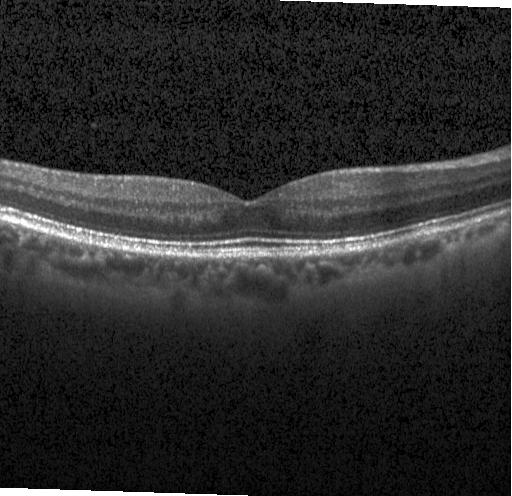

Optical coherence tomography B-scan, through the macula. Impression: no choroidal neovascularization, no diabetic macular edema, and no drusen.